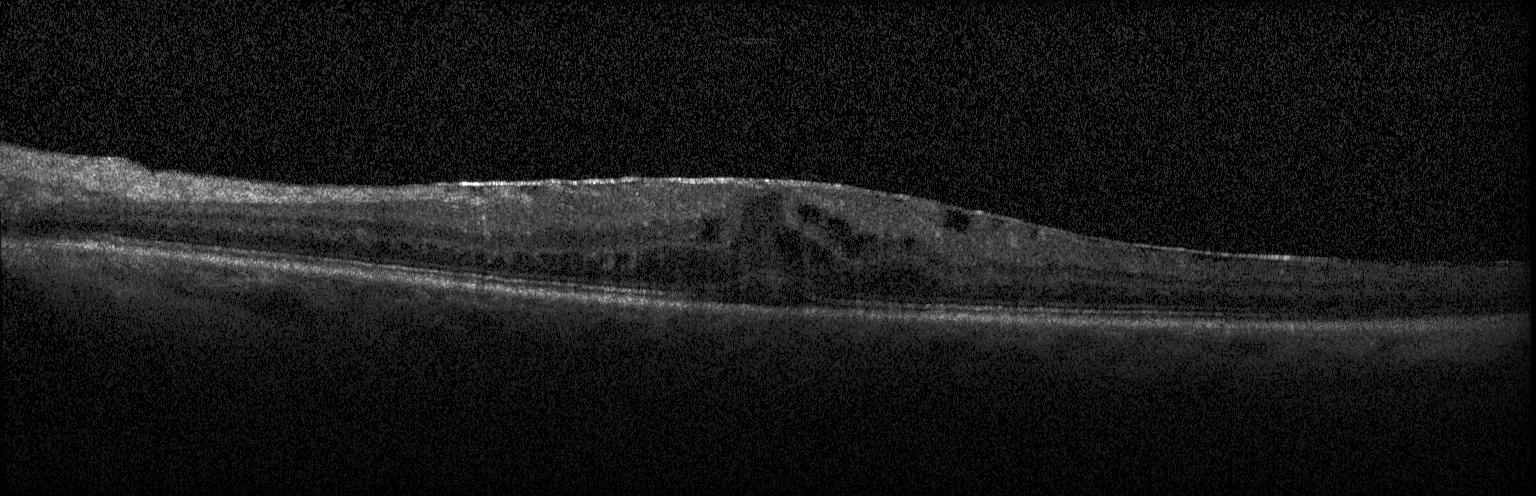 Optical coherence tomography scan, acquired on a Heidelberg Spectralis, through the macula — This B-scan demonstrates diabetic macular edema.